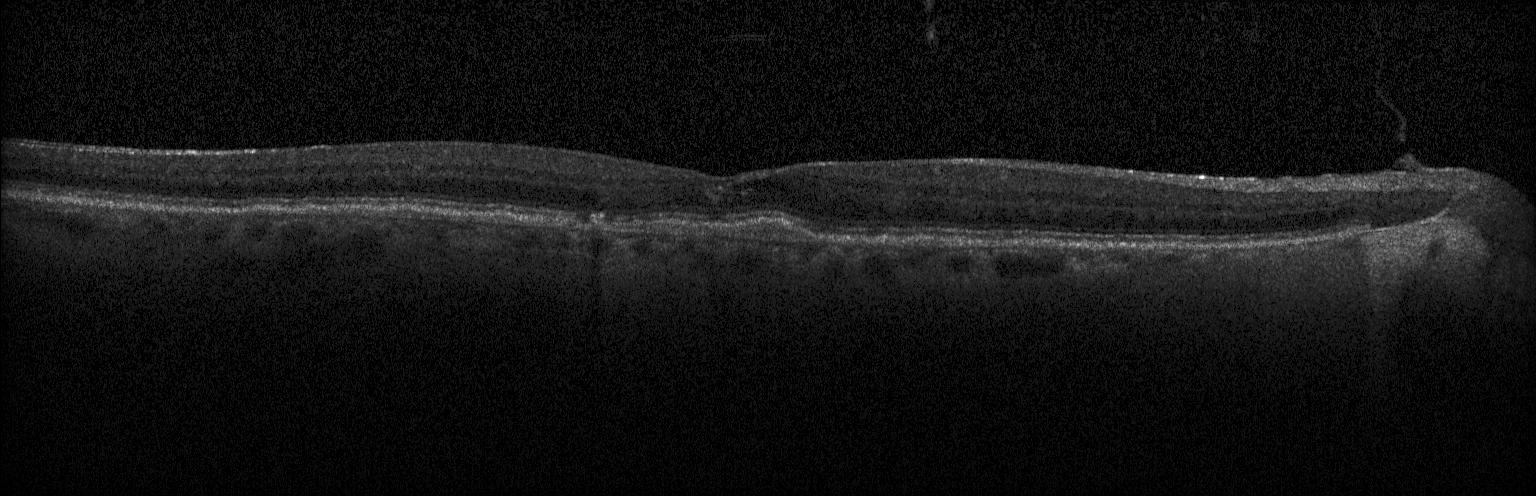 OCT scan showing choroidal neovascularization.